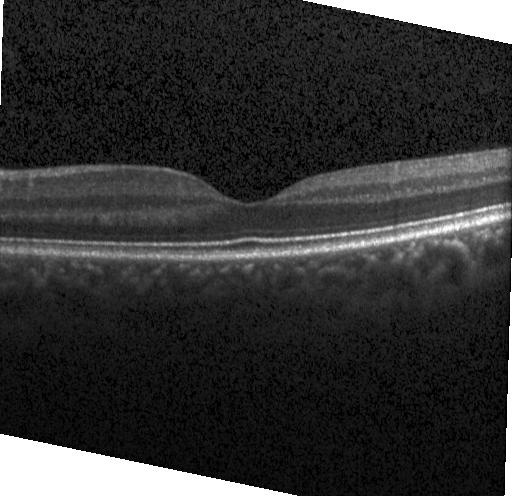
Spectral-domain OCT, optical coherence tomography scan. Dx: no evidence of CNV, DME, or drusen.